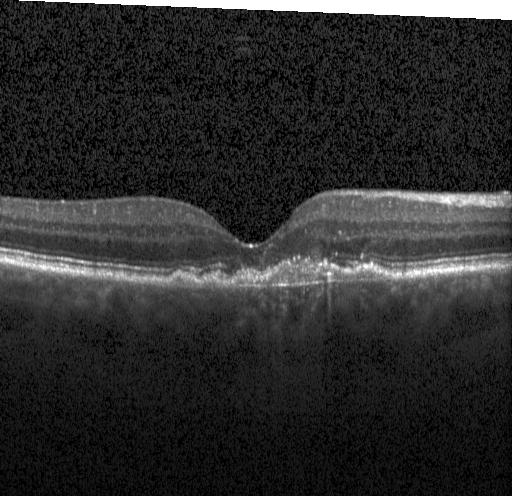 Fovea-centered. SD-OCT. Heidelberg Spectralis. Optical coherence tomography scan — Impression: CNV.